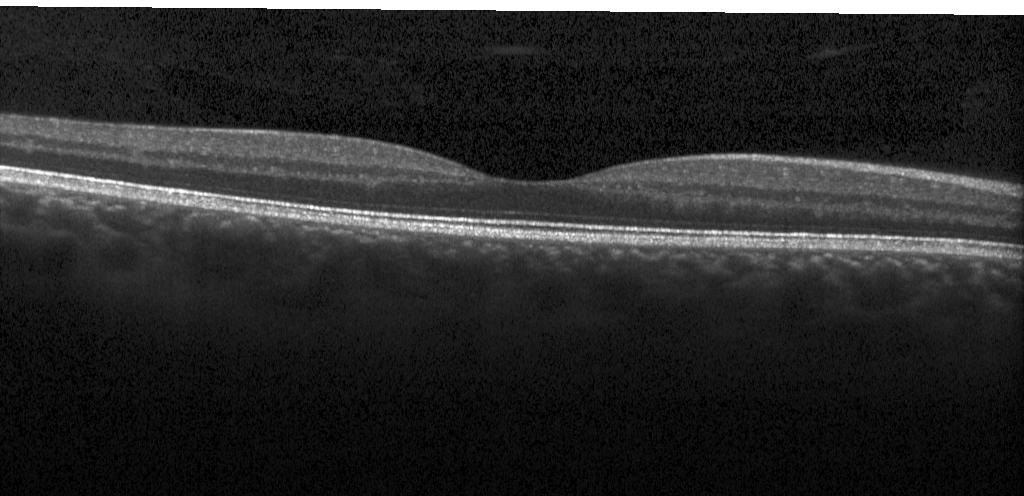 Finding: neither CNV, DME, nor drusen.